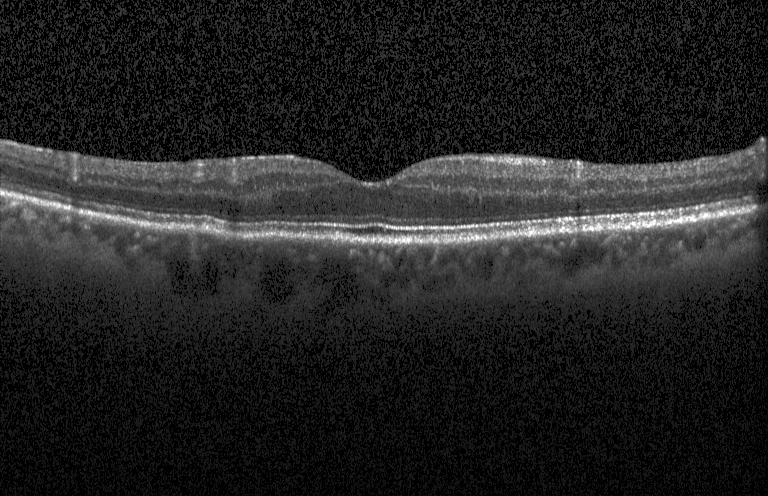

OCT B-scan
Diagnosis: no choroidal neovascularization, diabetic macular edema, or drusen.